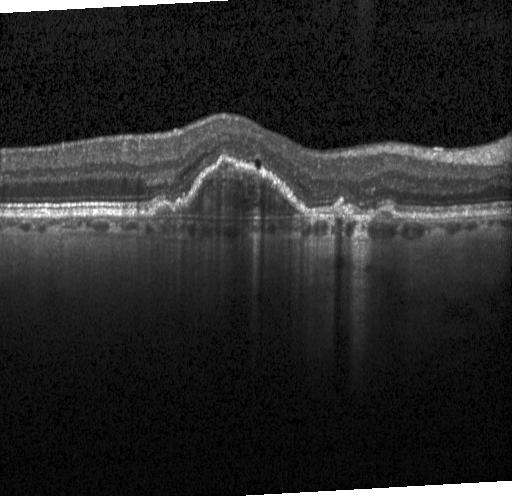
SD-OCT; OCT B-scan; Heidelberg Spectralis; fovea-centered.
A choroidal neovascular membrane.